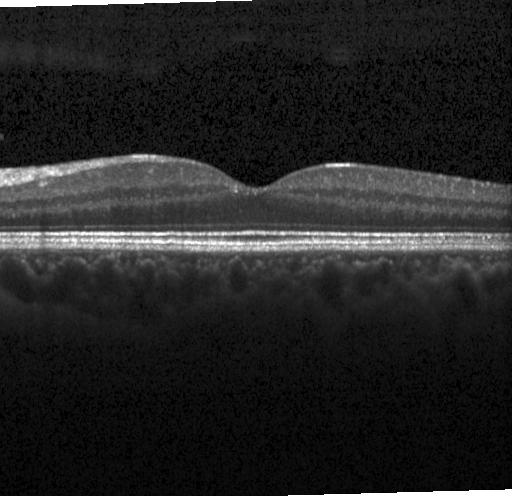

The scan shows no CNV, DME, or drusen.